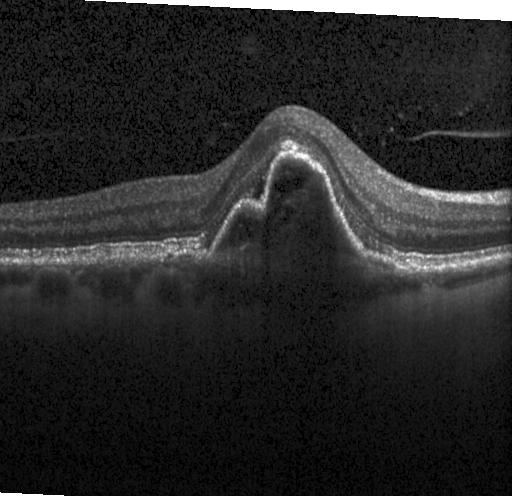
This B-scan demonstrates a choroidal neovascular membrane.